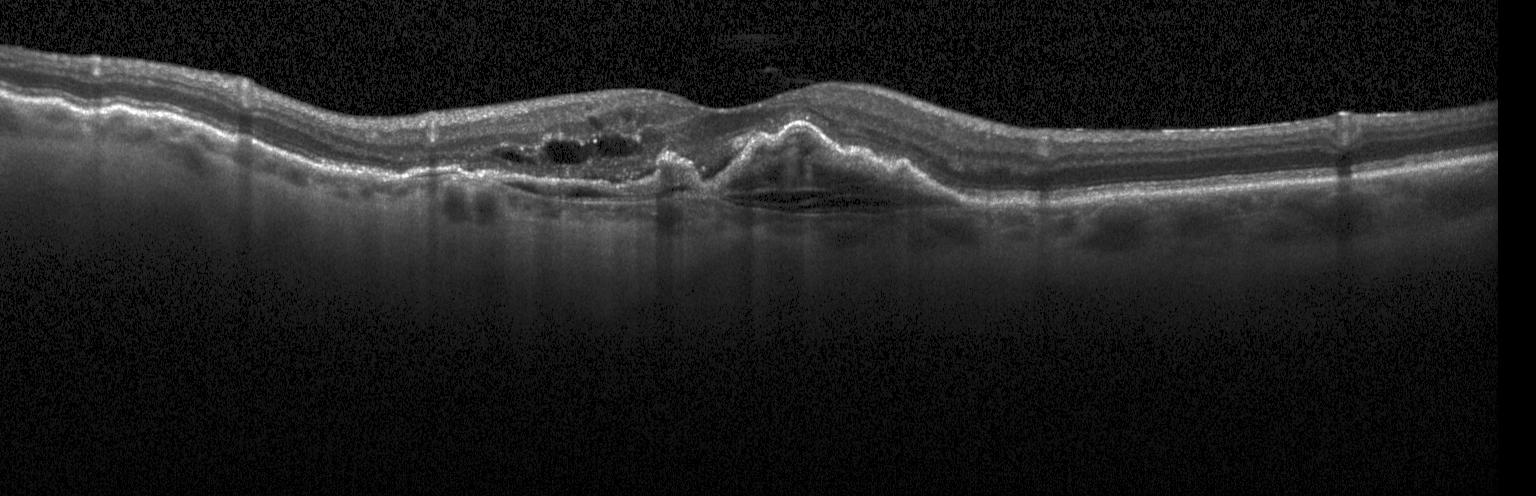
Optical coherence tomography B-scan
Dx: a choroidal neovascular membrane.